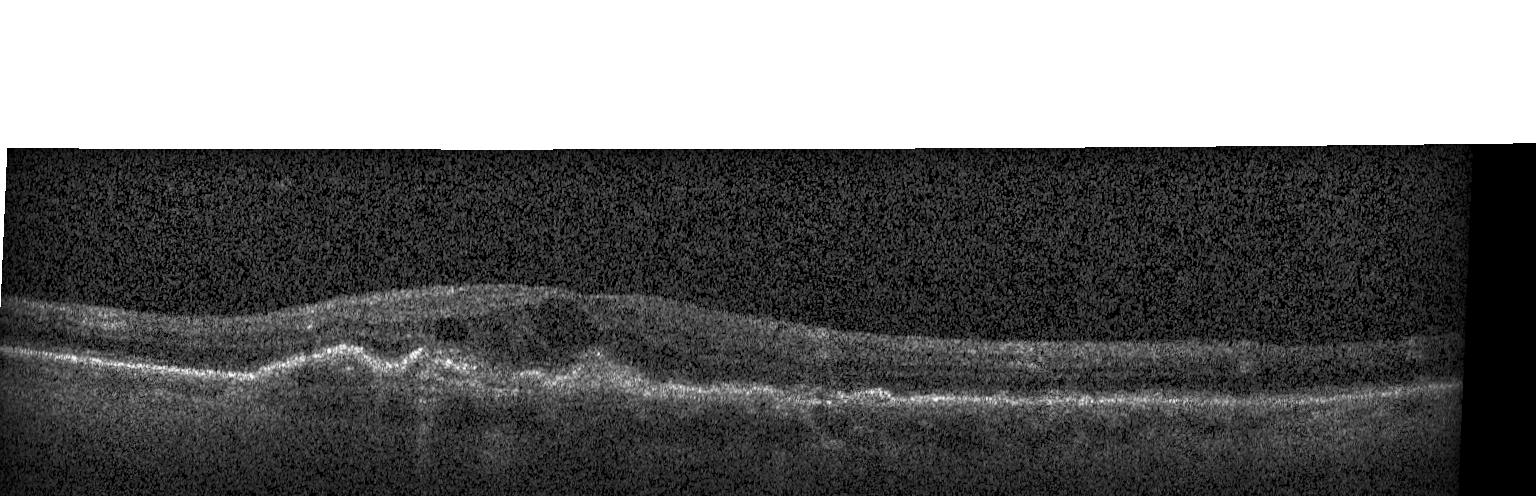

OCT B-scan. Macular OCT: CNV.